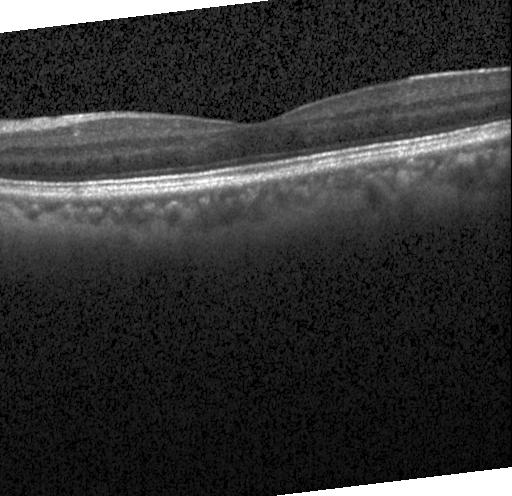 Optical coherence tomography B-scan · fovea-centered
The scan shows no CNV, no DME, and no drusen.